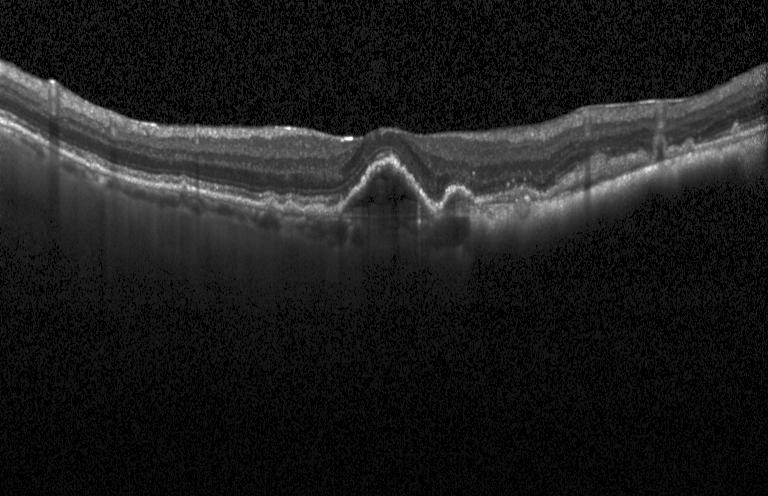
Fovea-centered. Retinal OCT B-scan.
Finding: a choroidal neovascular membrane.